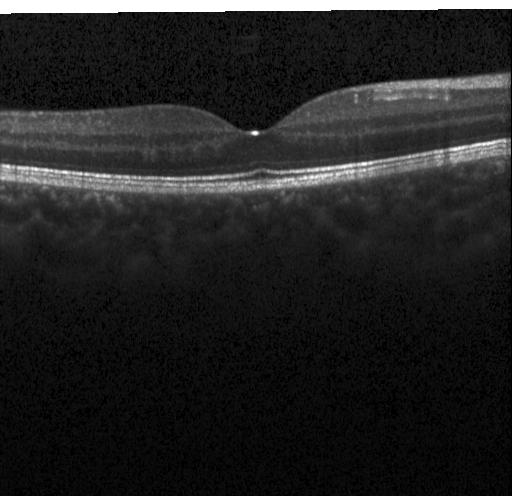

OCT scan showing no evidence of CNV, DME, or drusen.